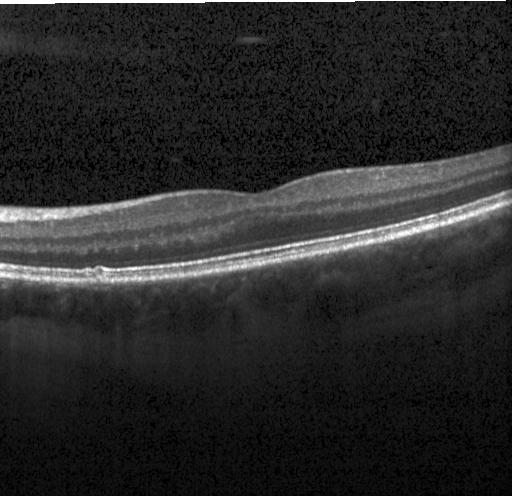 Heidelberg Spectralis OCT system, through the macula, optical coherence tomography scan, SD-OCT.
OCT finding: no choroidal neovascularization, diabetic macular edema, or drusen.